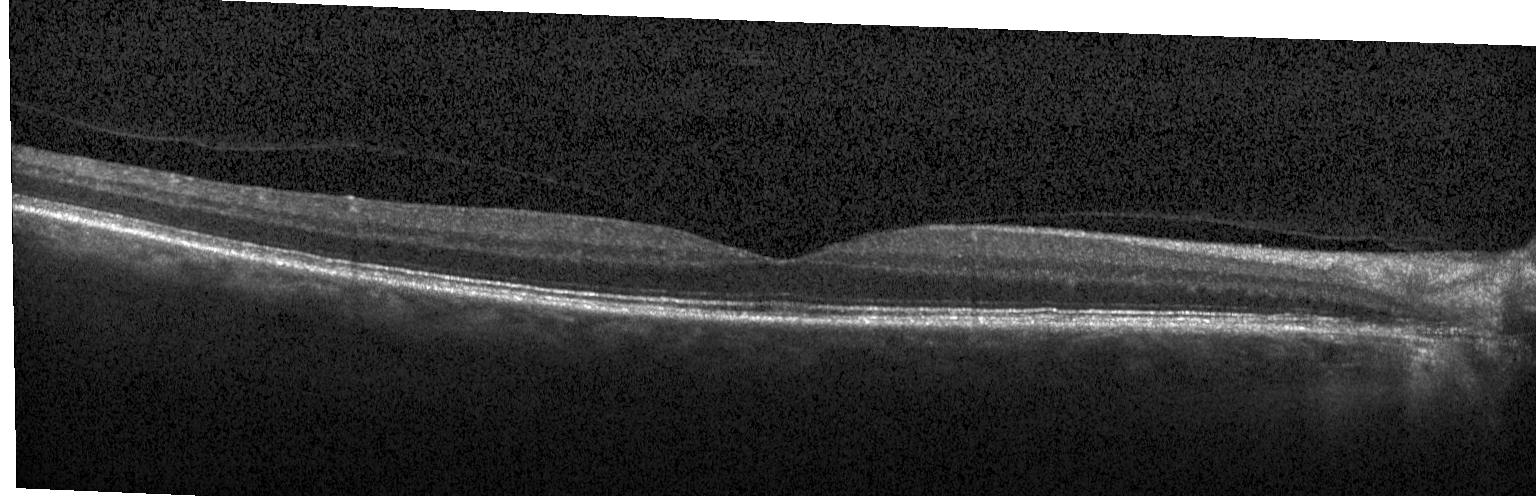 OCT line scan, Heidelberg Spectralis OCT system, SD-OCT, macular scan
Dx: no choroidal neovascularization, diabetic macular edema, or drusen.